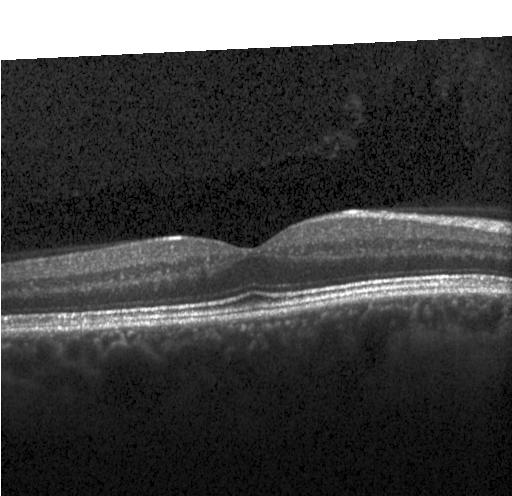
This B-scan demonstrates no evidence of choroidal neovascularization, diabetic macular edema, or drusen.